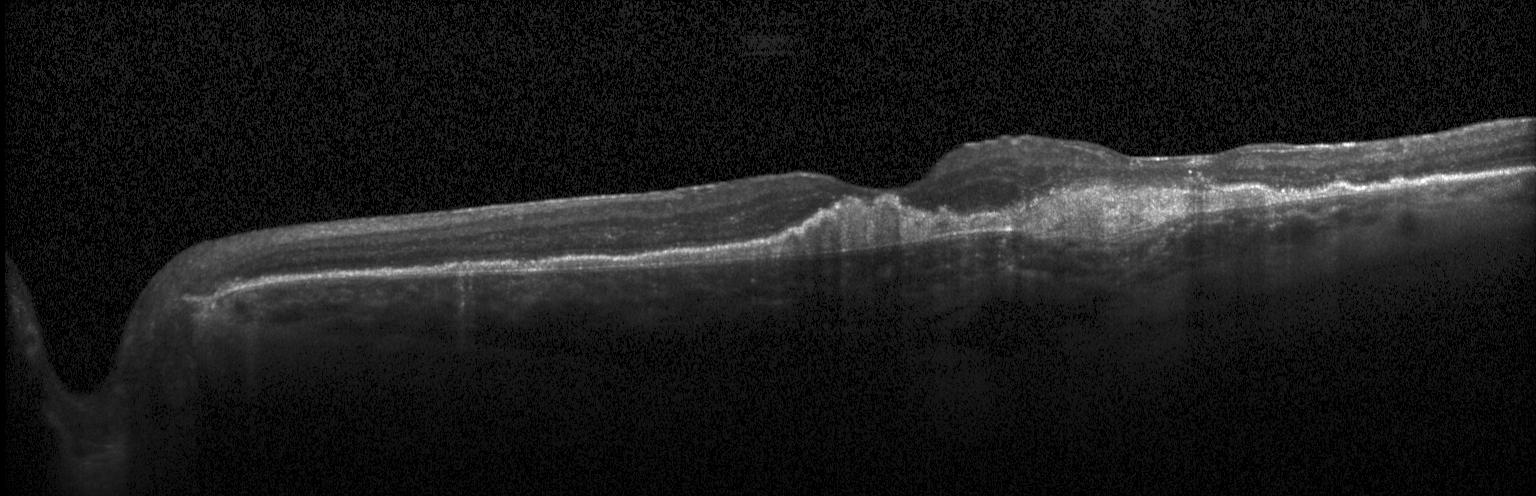
Spectral-domain OCT B-scan: CNV.